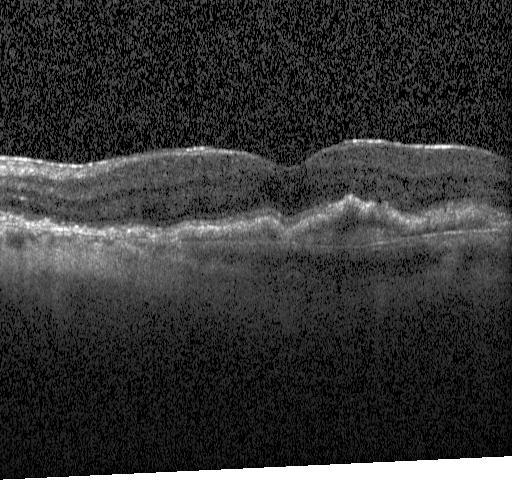 Macular OCT: a choroidal neovascular membrane.